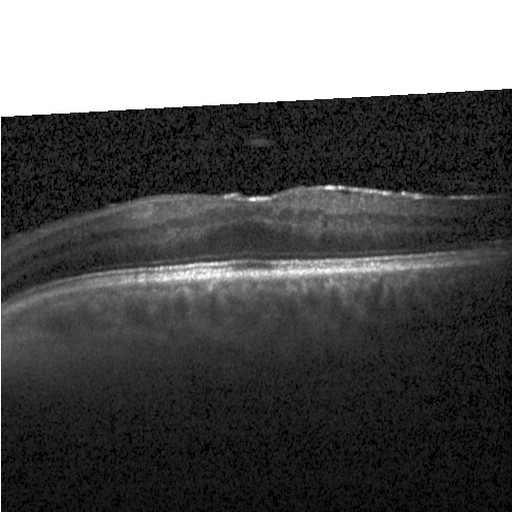

Horizontal scan through the fovea · SD-OCT · Heidelberg Spectralis OCT system · OCT B-scan — OCT finding: DME.